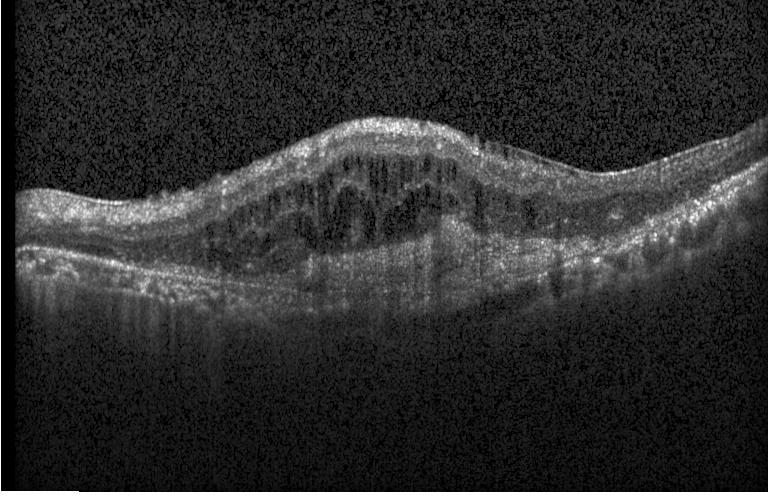
Finding: a choroidal neovascular membrane.